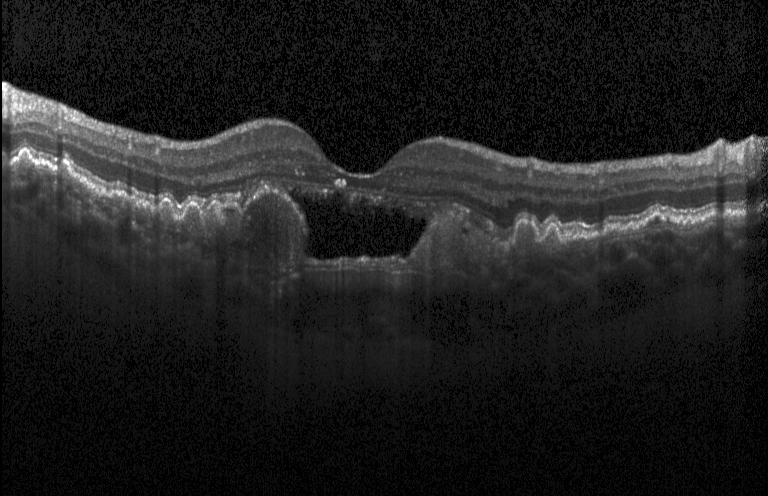

Diagnosis: choroidal neovascularization.